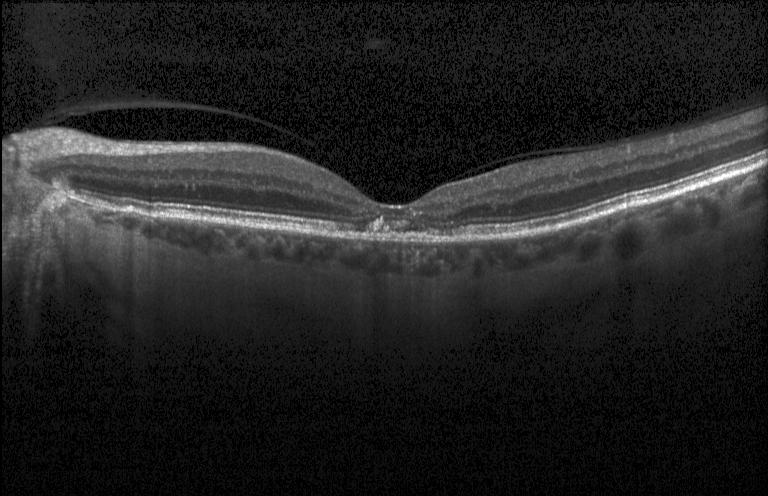
Optical coherence tomography scan, Heidelberg Spectralis. The scan shows choroidal neovascularization (CNV).